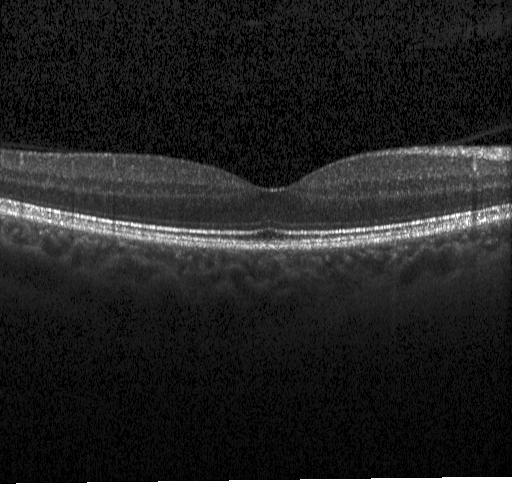

OCT line scan. This B-scan demonstrates no CNV, no DME, and no drusen.